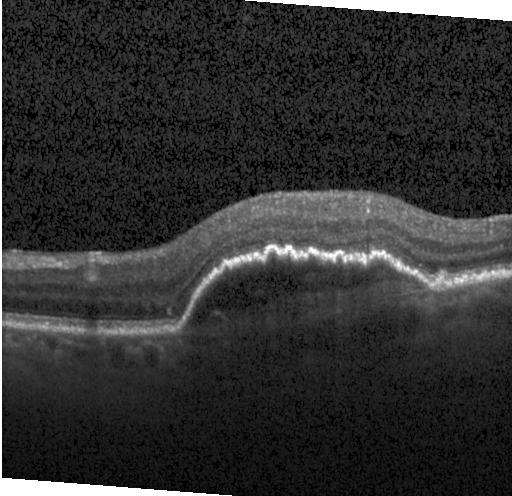

Heidelberg Spectralis. SD-OCT. Centered on the fovea. Optical coherence tomography scan
The scan shows choroidal neovascularization.